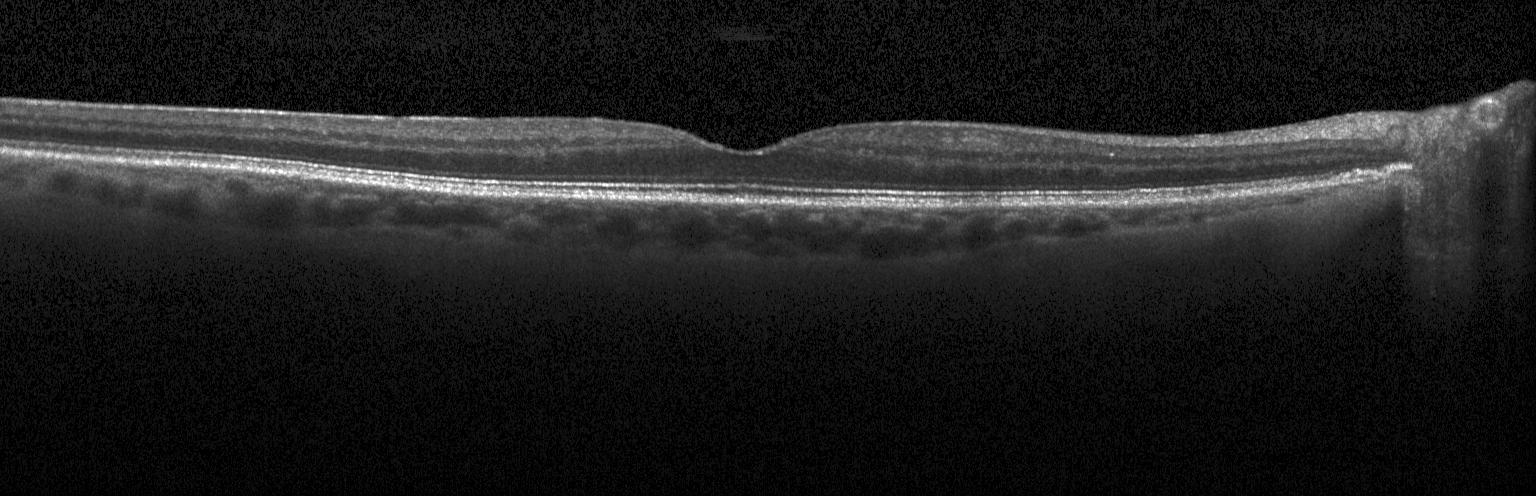 Optical coherence tomography B-scan — Impression: neither choroidal neovascularization, diabetic macular edema, nor drusen.